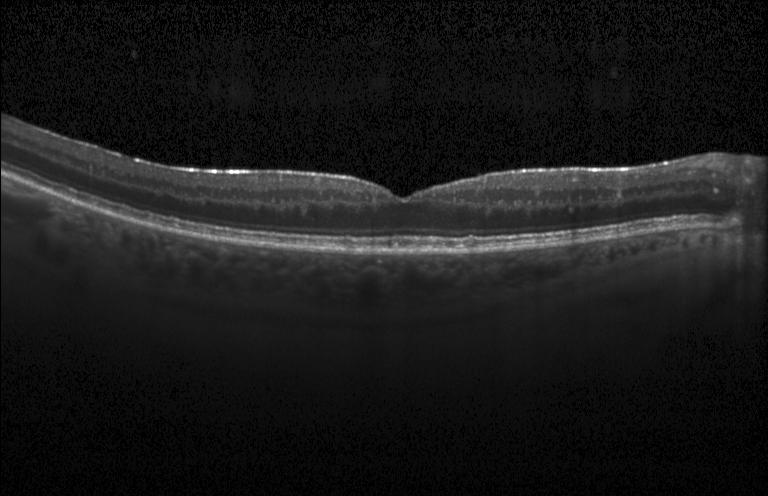 OCT line scan; spectral-domain OCT; horizontal scan through the fovea — OCT finding: no CNV, DME, or drusen.